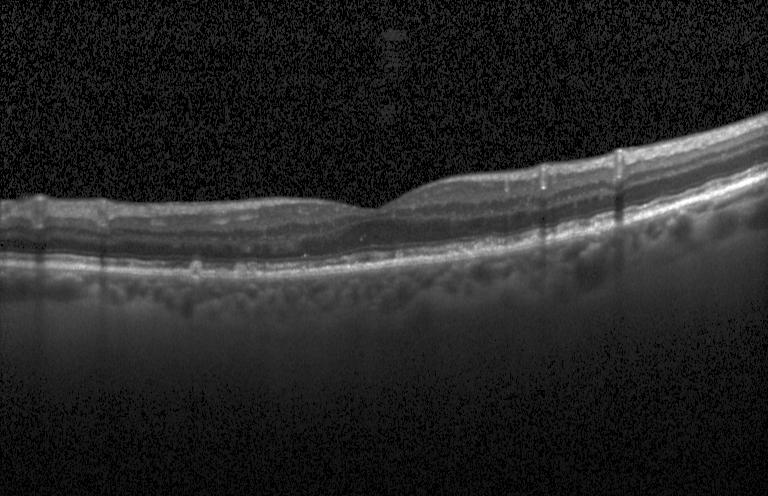

OCT scan showing drusen.